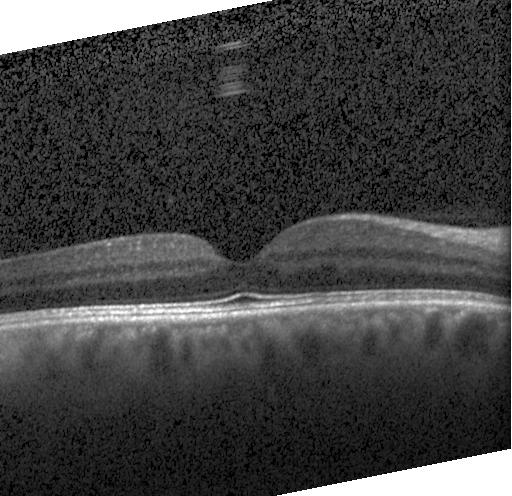
Acquired on a Heidelberg Spectralis, macular scan, spectral-domain optical coherence tomography, retinal OCT B-scan
Diagnosis: no evidence of CNV, DME, or drusen.